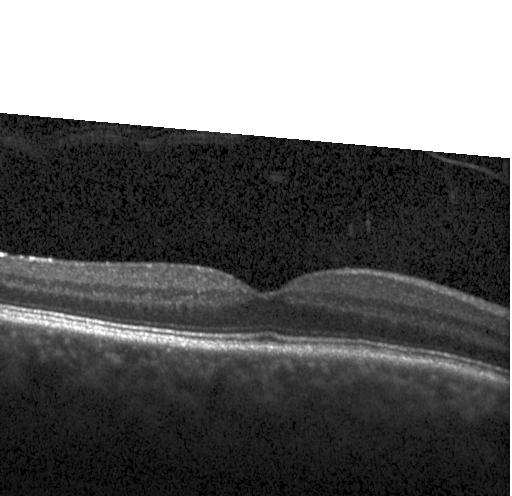

This B-scan demonstrates neither choroidal neovascularization, diabetic macular edema, nor drusen.